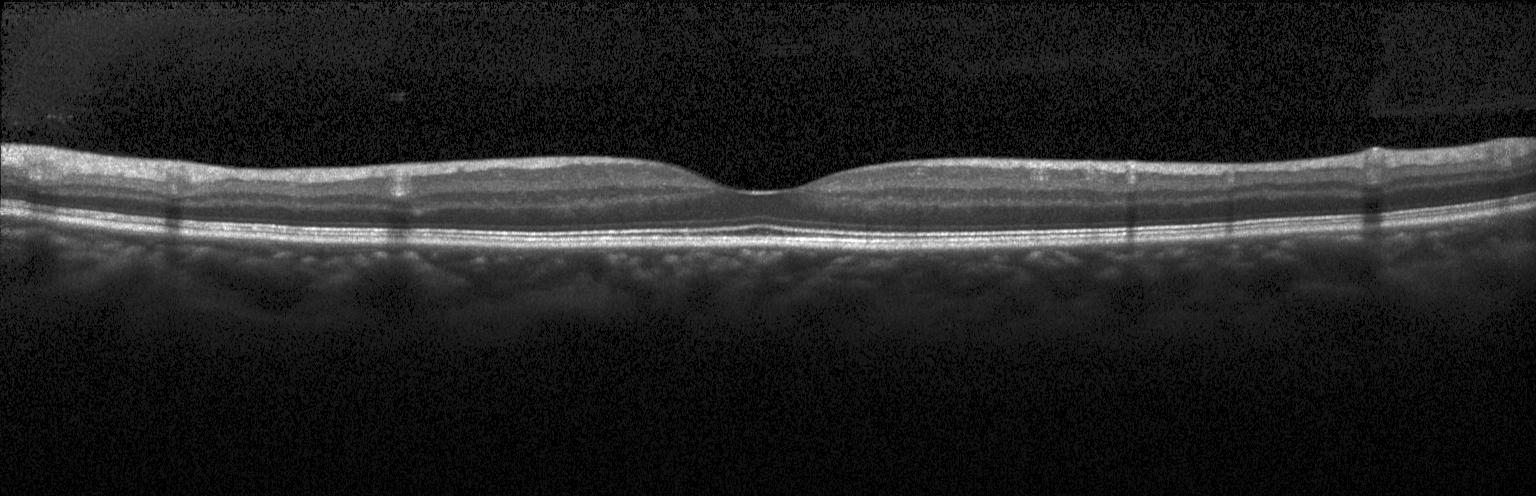
Spectral-domain OCT. Centered on the fovea. Retinal OCT B-scan. Heidelberg Spectralis. This B-scan demonstrates no choroidal neovascularization, diabetic macular edema, or drusen.